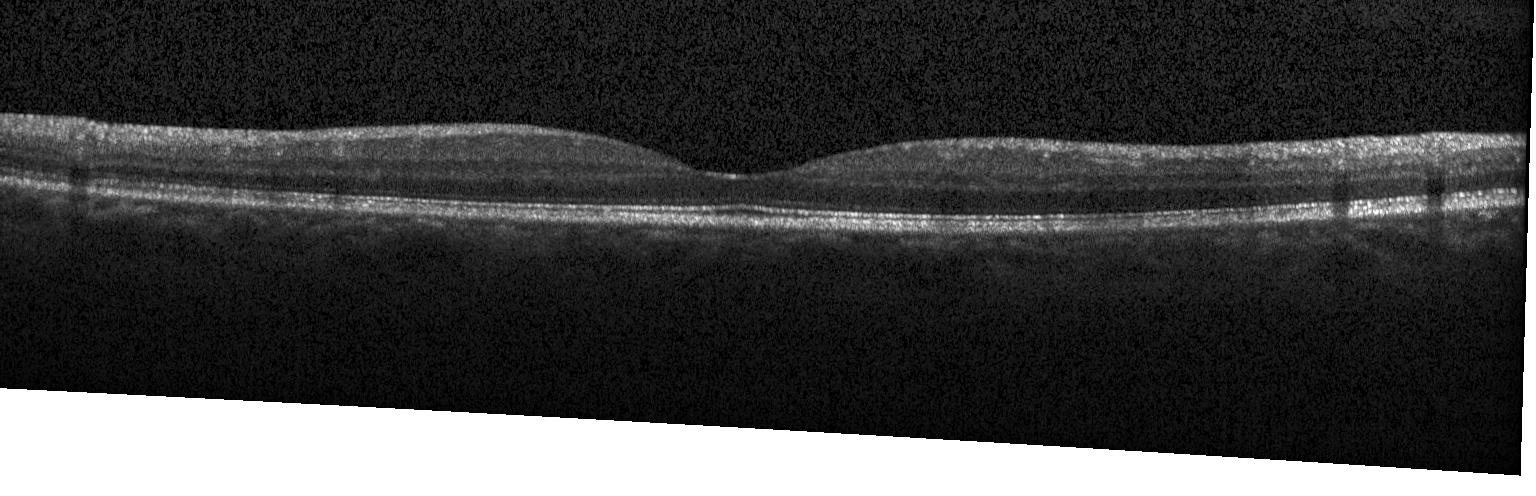 The scan shows no evidence of CNV, DME, or drusen.